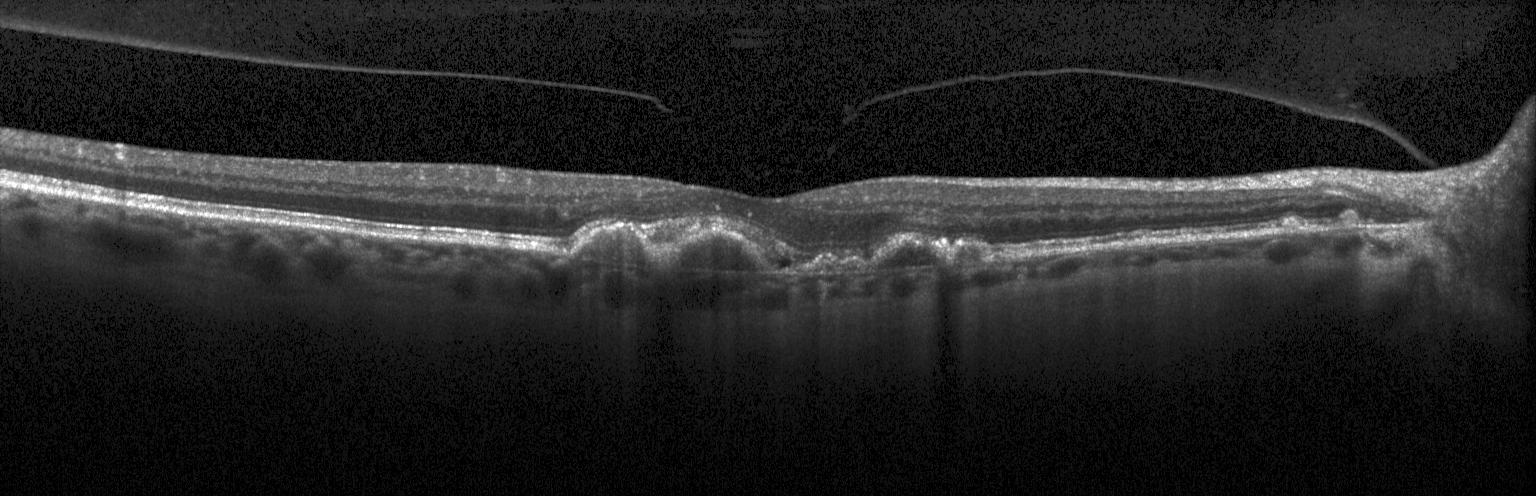
Retinal OCT B-scan, fovea-centered, spectral-domain optical coherence tomography
Choroidal neovascularization.